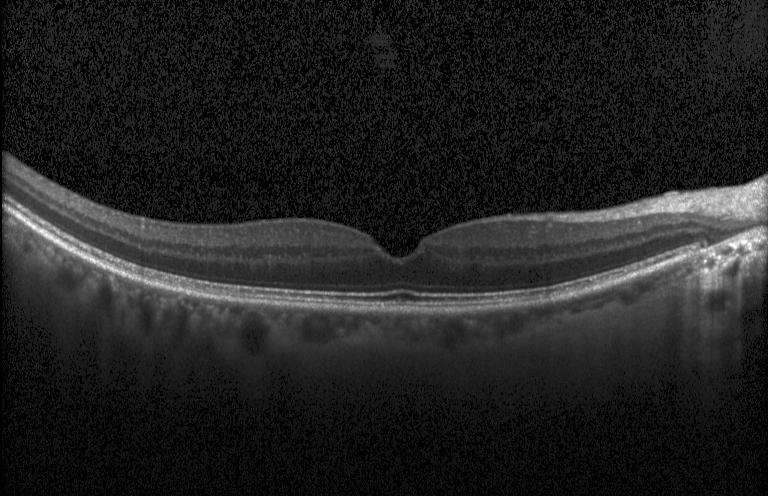

Acquired on a Heidelberg Spectralis · fovea-centered · retinal OCT B-scan · spectral-domain OCT — Assessment: no evidence of choroidal neovascularization, diabetic macular edema, or drusen.